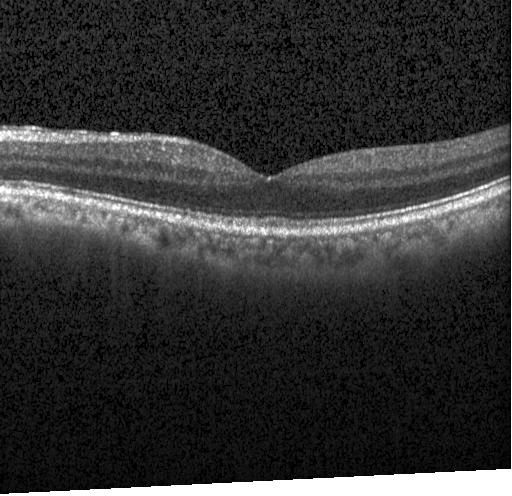
Finding: no choroidal neovascularization, no diabetic macular edema, and no drusen.